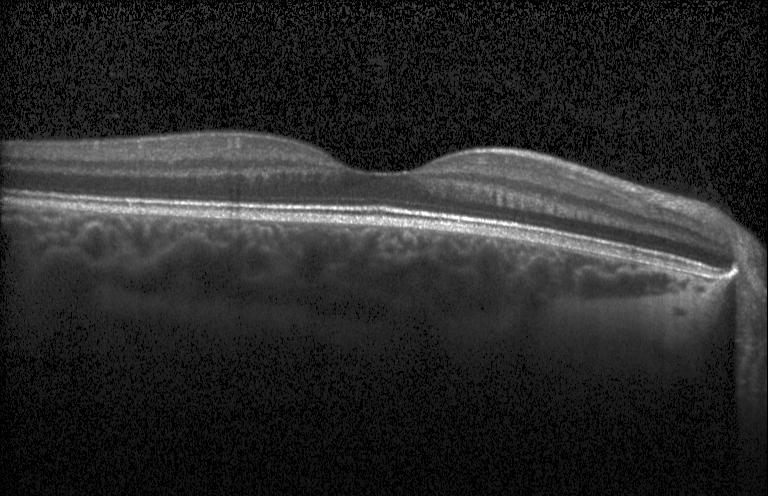
Dx: no evidence of CNV, DME, or drusen.